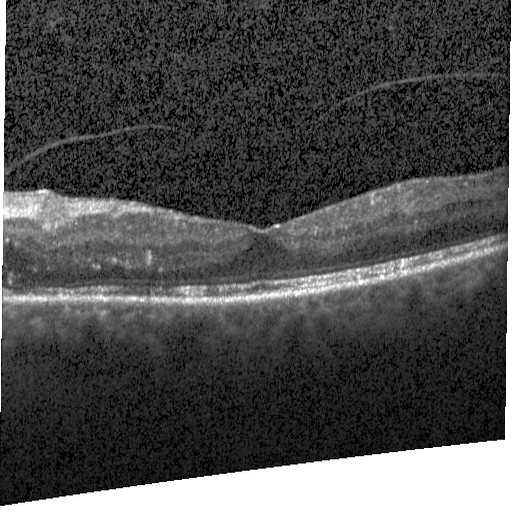 Macular OCT demonstrating diabetic macular edema.